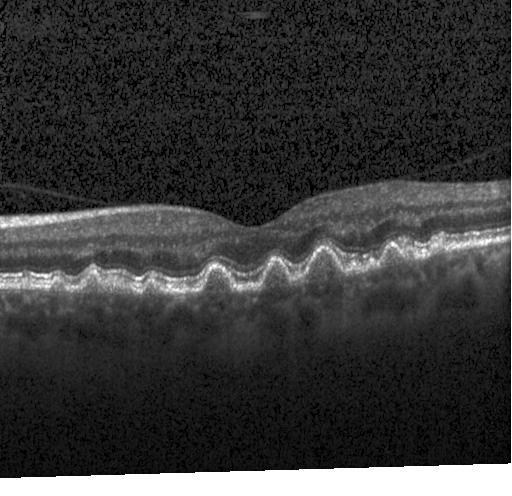 Diagnosis: multiple drusen.